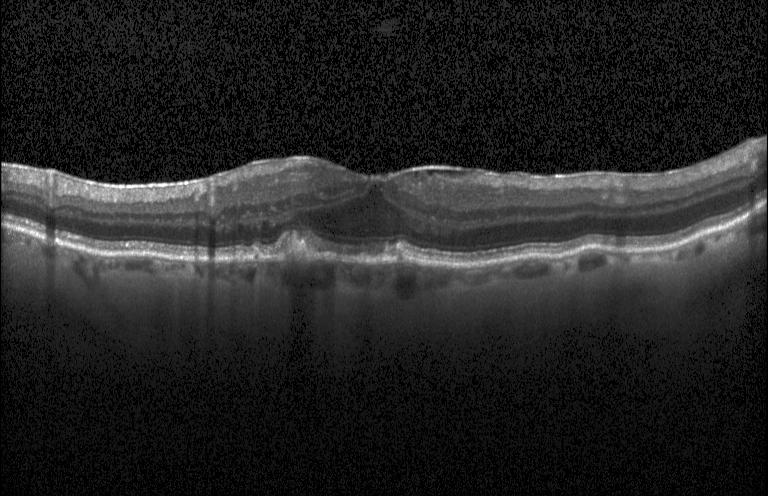

Acquired on a Heidelberg Spectralis, SD-OCT, retinal OCT B-scan — This B-scan demonstrates choroidal neovascularization (CNV).